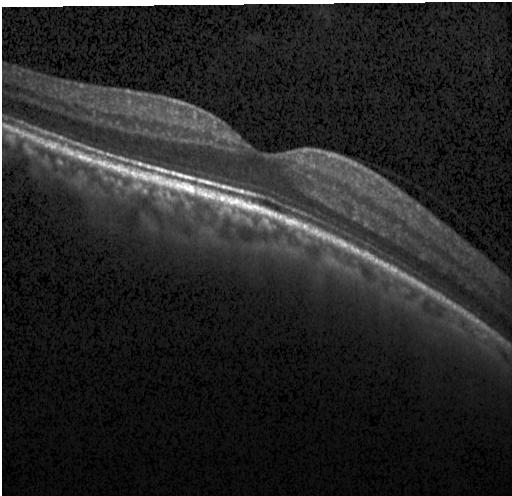
OCT finding: no choroidal neovascularization, no diabetic macular edema, and no drusen.